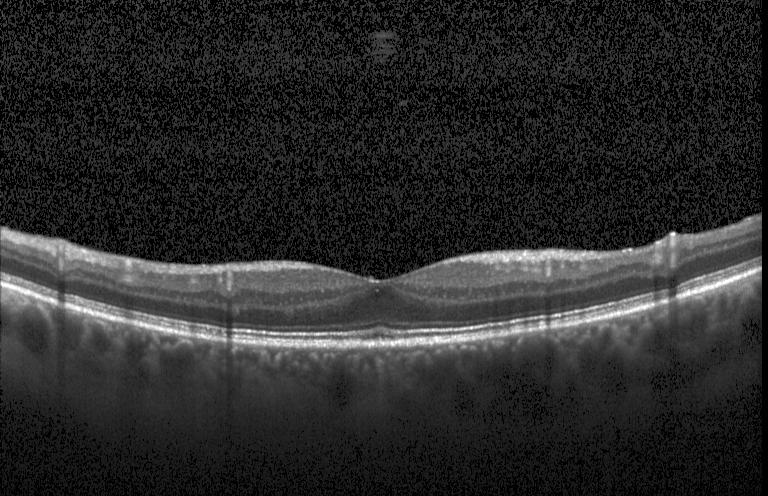 SD-OCT; OCT B-scan; Heidelberg Spectralis. Macular OCT: no CNV, DME, or drusen.